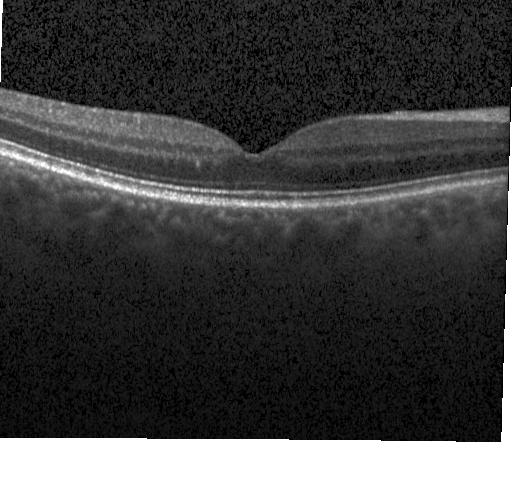

Spectral-domain OCT. Optical coherence tomography scan. Centered on the fovea.
Diagnosis: no CNV, DME, or drusen.